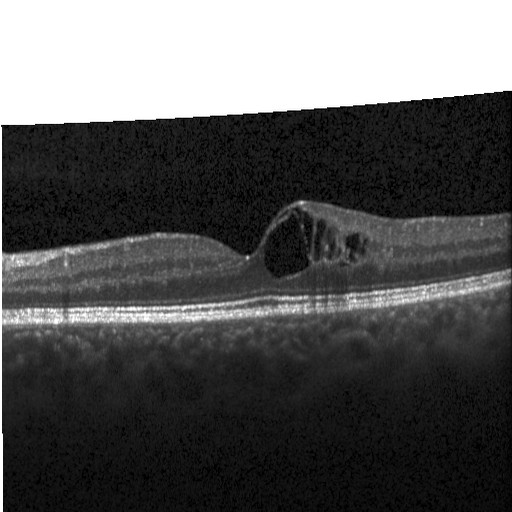

Assessment: diabetic macular edema.